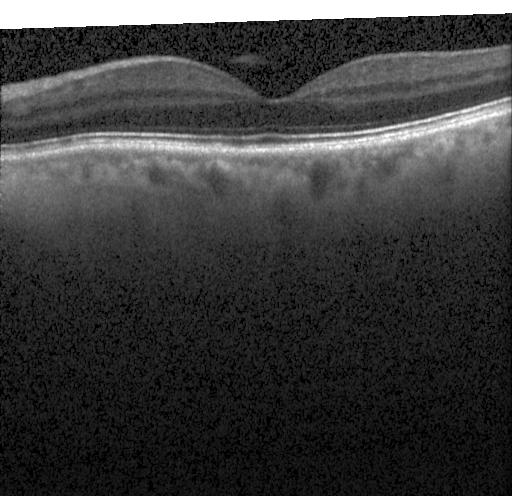 Macular OCT: no CNV, no DME, and no drusen.